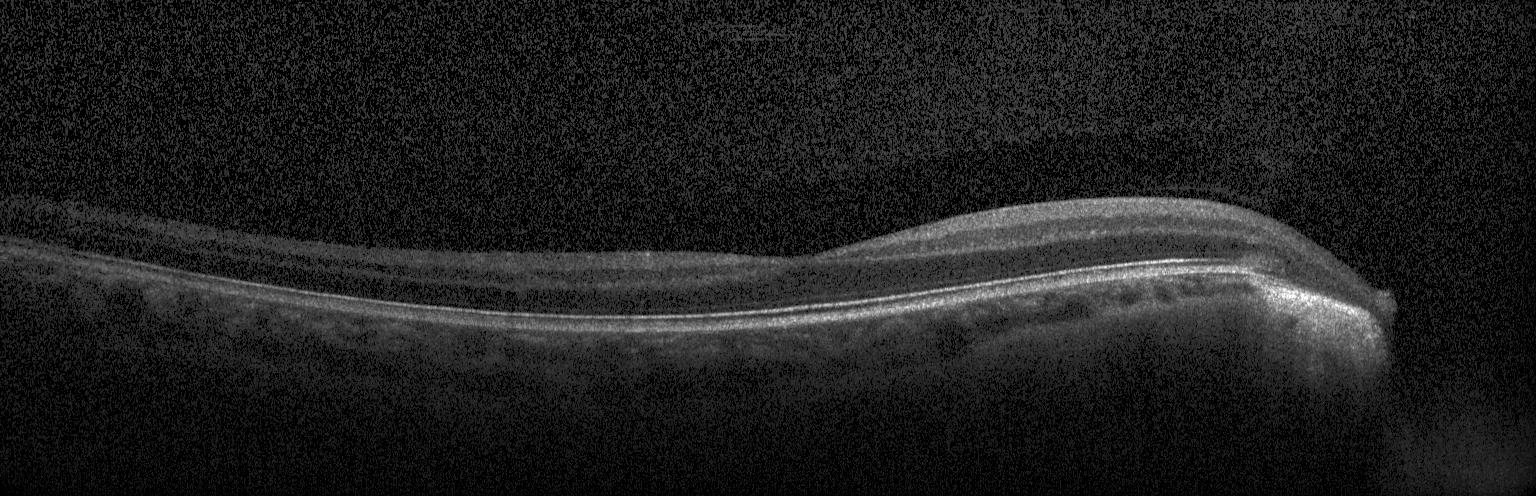 The scan shows neither CNV, DME, nor drusen.